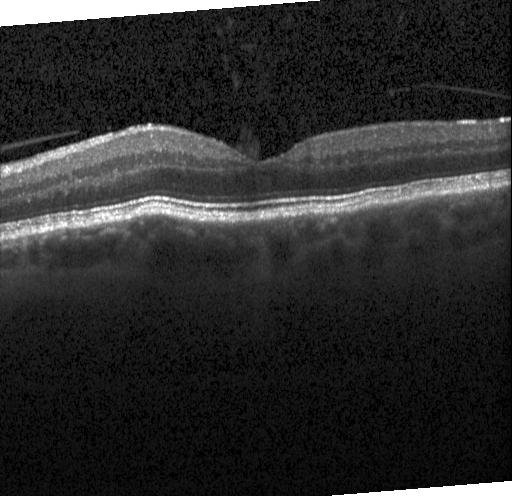

Diagnosis: no choroidal neovascularization, no diabetic macular edema, and no drusen.